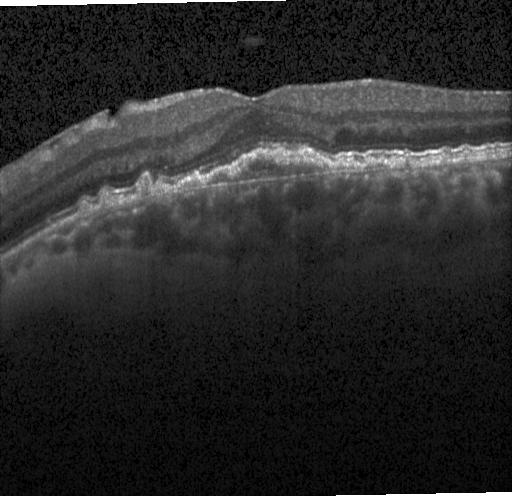 Spectral-domain optical coherence tomography · fovea-centered · Heidelberg Spectralis OCT system · optical coherence tomography scan.
Macular OCT: choroidal neovascularization (CNV).